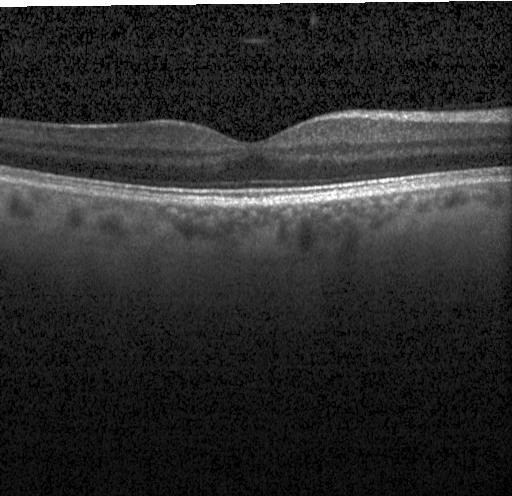 Macular scan, spectral-domain optical coherence tomography, Heidelberg Spectralis, OCT line scan — Dx: no CNV, no DME, and no drusen.